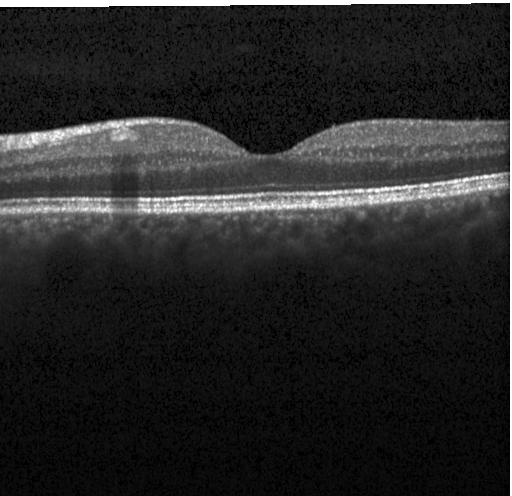 Retinal OCT B-scan — Assessment: no evidence of choroidal neovascularization, diabetic macular edema, or drusen.